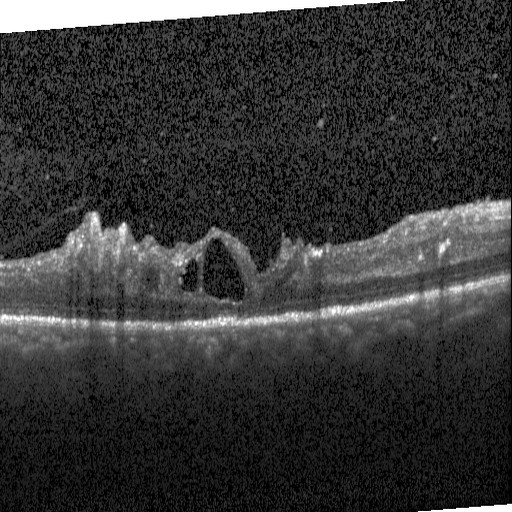

Impression: DME.